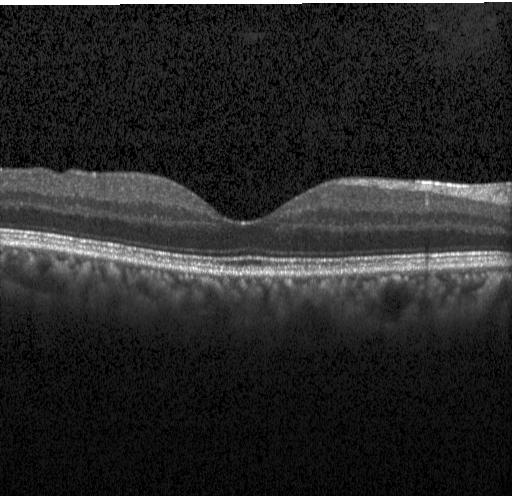

Retinal OCT cross-section · Heidelberg Spectralis OCT system — OCT finding: no evidence of choroidal neovascularization, diabetic macular edema, or drusen.